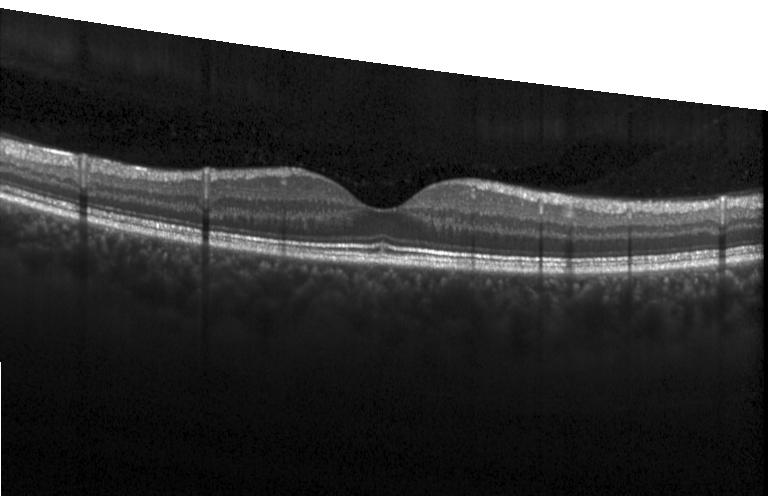

Dx: no choroidal neovascularization, diabetic macular edema, or drusen.